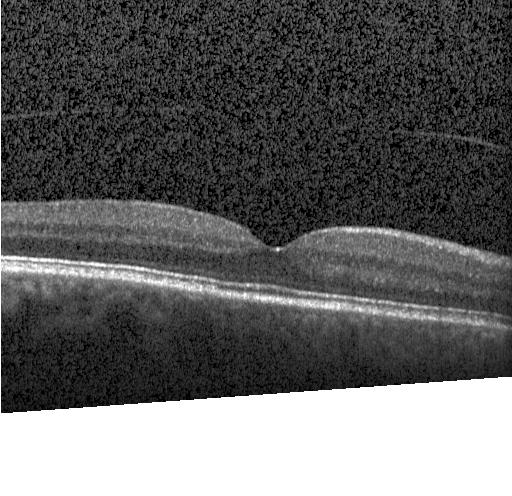
Retinal OCT B-scan. Diagnosis: no CNV, DME, or drusen.